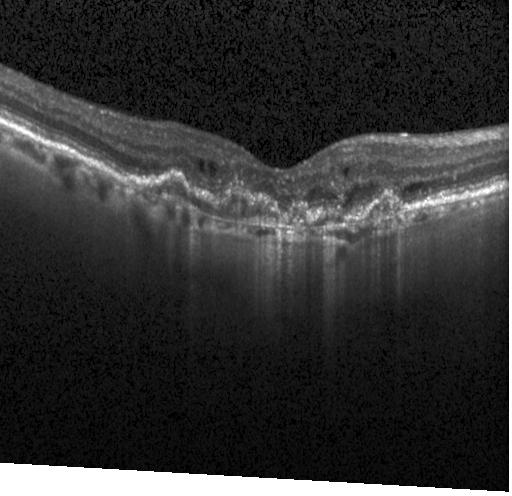

Heidelberg Spectralis OCT system, OCT line scan, spectral-domain OCT, macular scan. Macular OCT: a choroidal neovascular membrane.